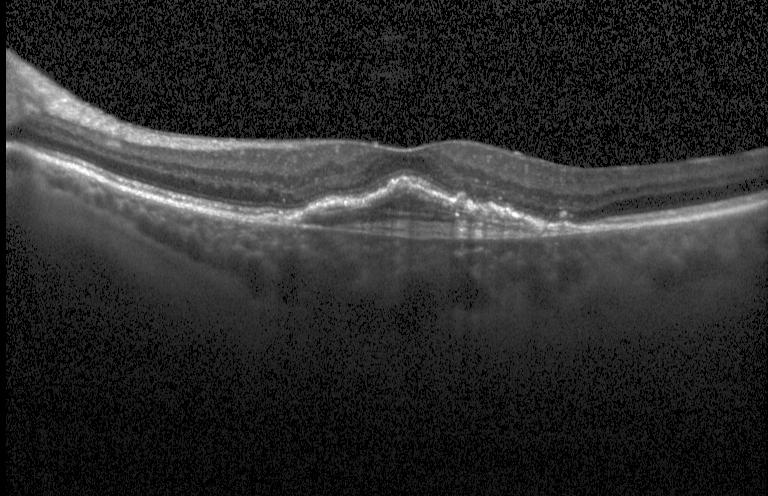
Optical coherence tomography scan
Diagnosis: a choroidal neovascular membrane.